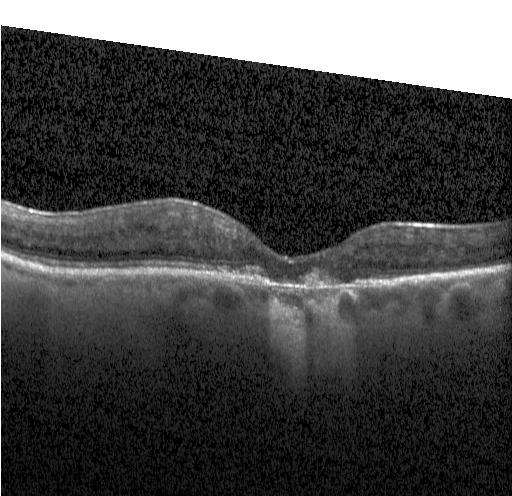

OCT line scan.
Diagnosis: a choroidal neovascular membrane.